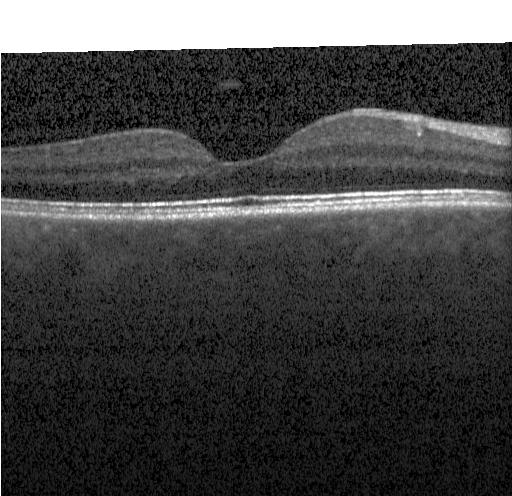

Macular scan · optical coherence tomography B-scan.
Finding: neither CNV, DME, nor drusen.